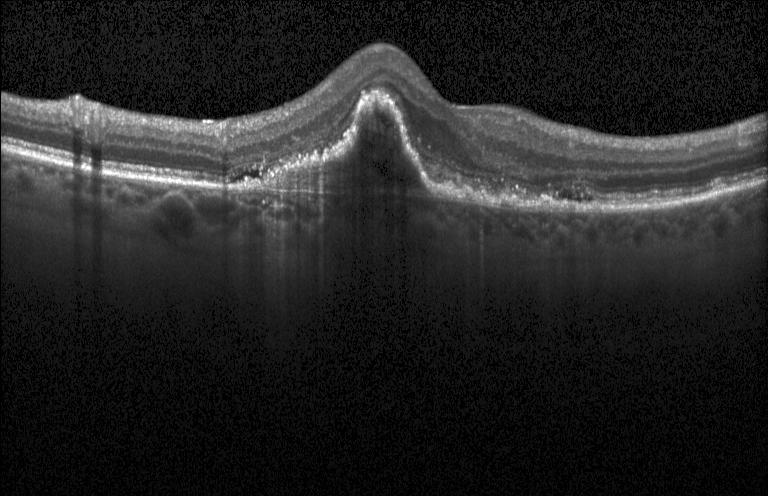 This B-scan demonstrates choroidal neovascularization (CNV).